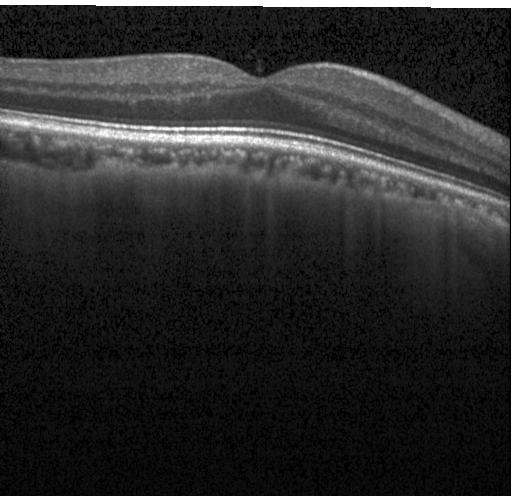 Fovea-centered. OCT line scan — Impression: neither CNV, DME, nor drusen.